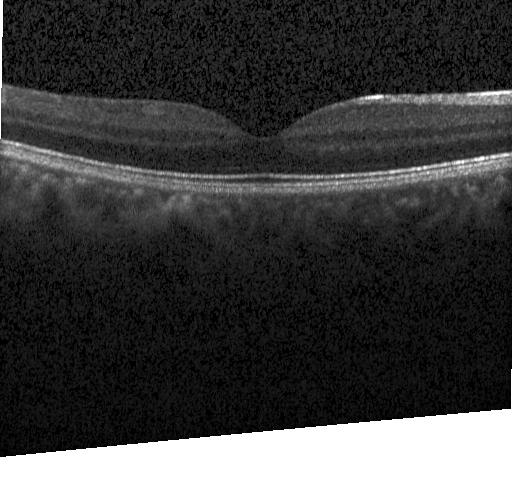 OCT B-scan showing neither choroidal neovascularization, diabetic macular edema, nor drusen.